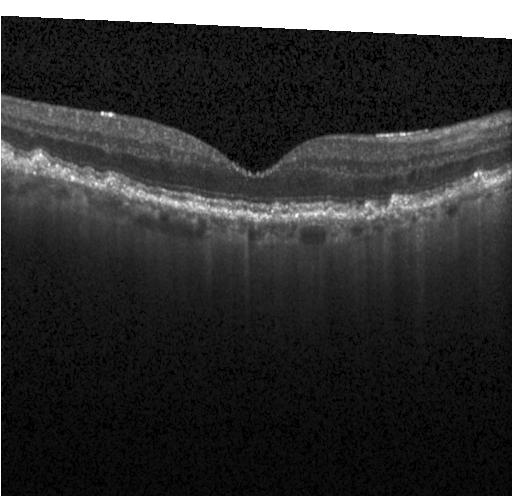 Retinal OCT cross-section — Finding: drusen.